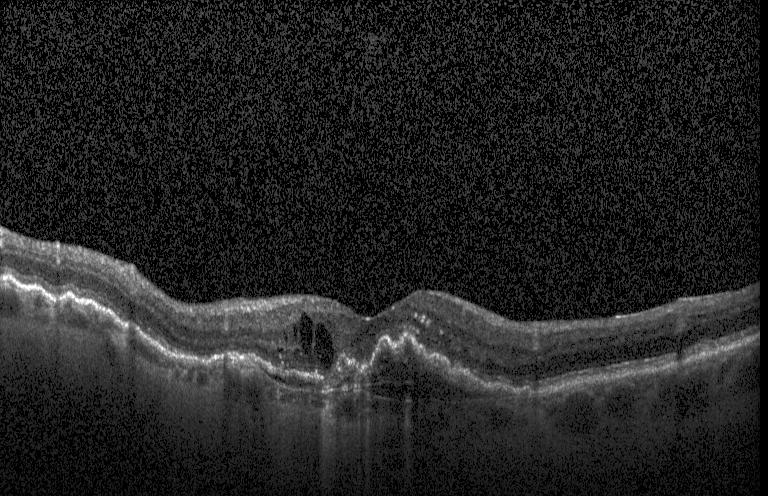

OCT B-scan
This B-scan demonstrates a choroidal neovascular membrane.